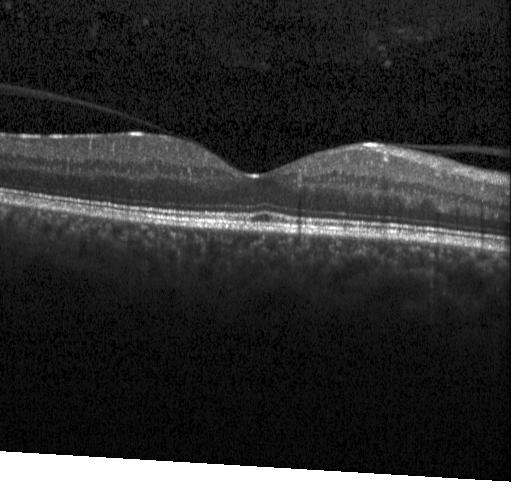

Diagnosis: no choroidal neovascularization, diabetic macular edema, or drusen.